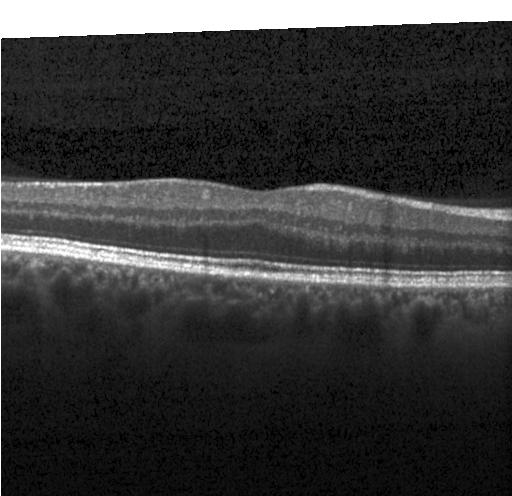
Macular scan. OCT line scan — OCT finding: no evidence of CNV, DME, or drusen.